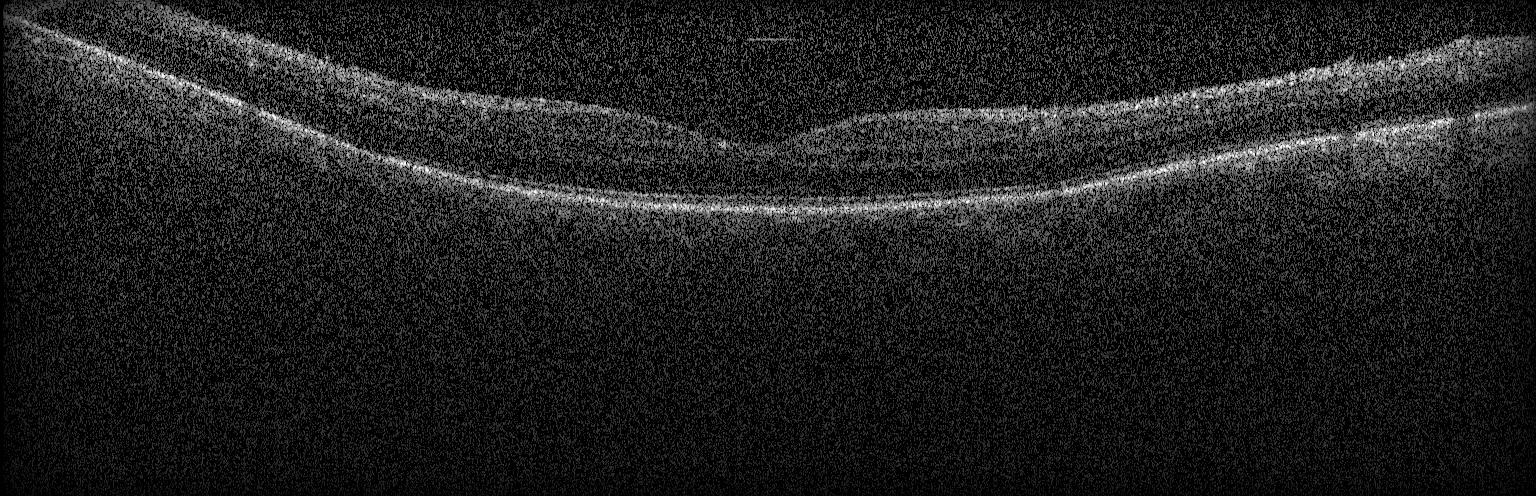

The scan shows no evidence of choroidal neovascularization, diabetic macular edema, or drusen.